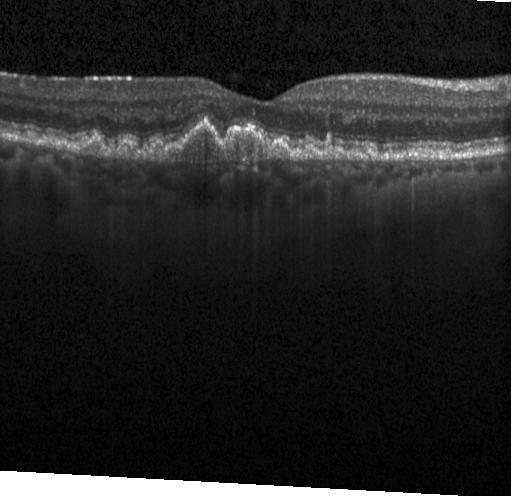 Impression: choroidal neovascularization.